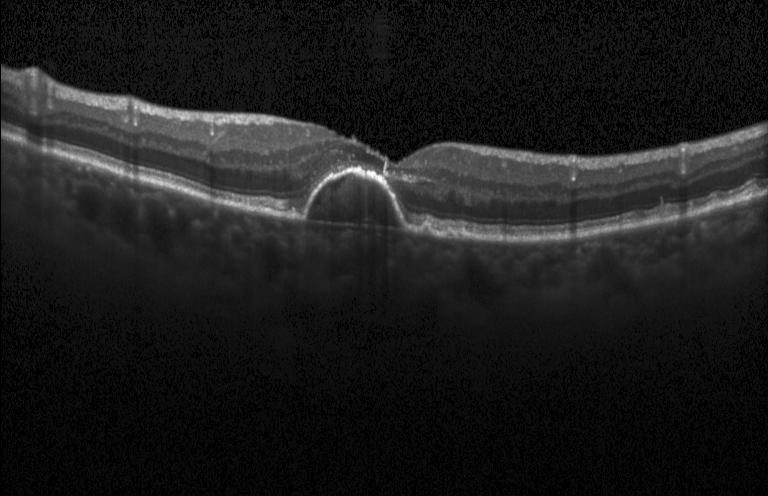

Retinal OCT cross-section showing CNV.